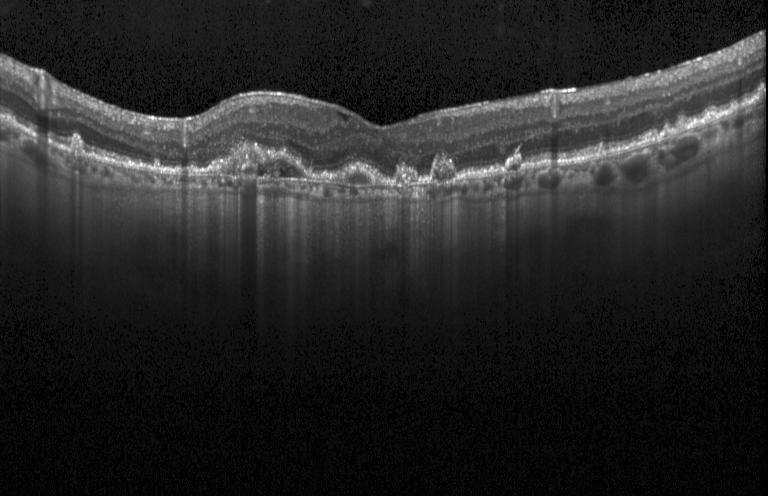 Through the macula · retinal OCT B-scan · spectral-domain optical coherence tomography · acquired on a Heidelberg Spectralis
Impression: a choroidal neovascular membrane.